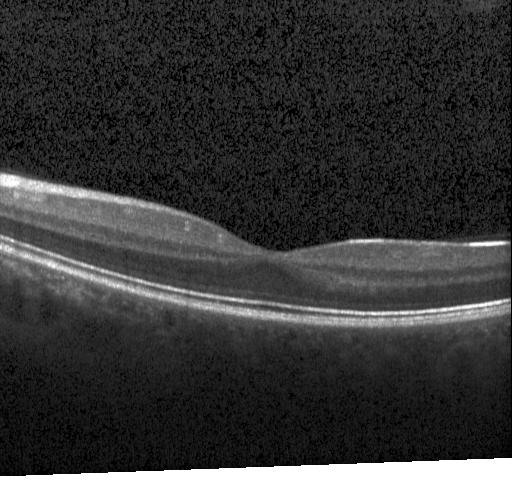
Diagnosis: no evidence of CNV, DME, or drusen.